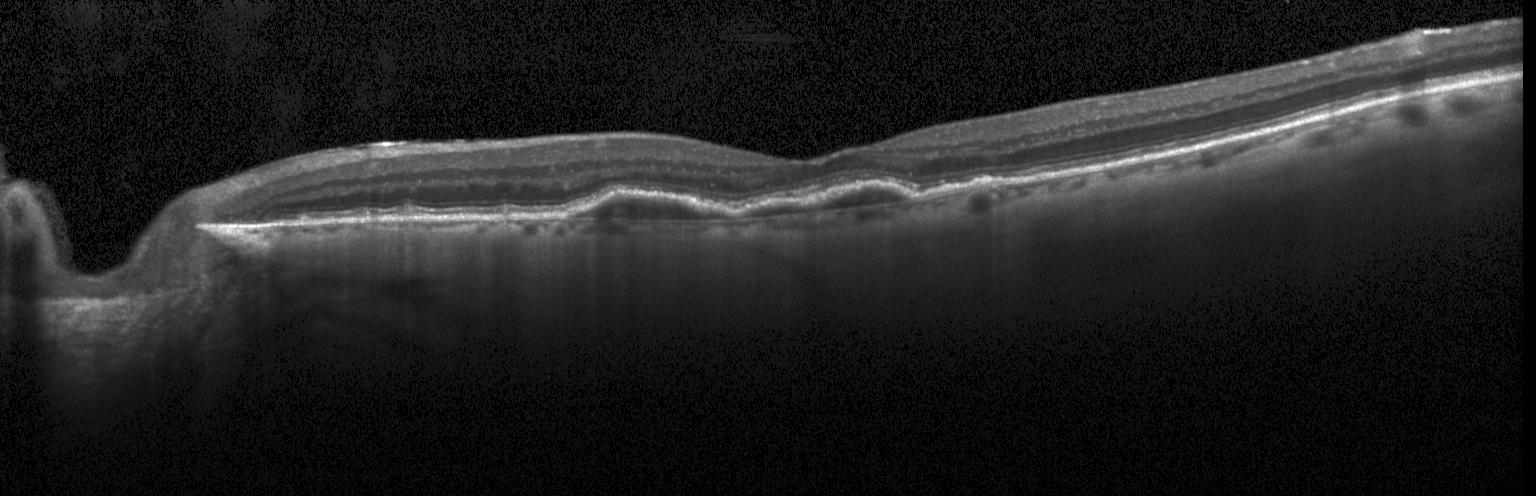
Instrument: Heidelberg Spectralis; OCT line scan
Impression: choroidal neovascularization (CNV).